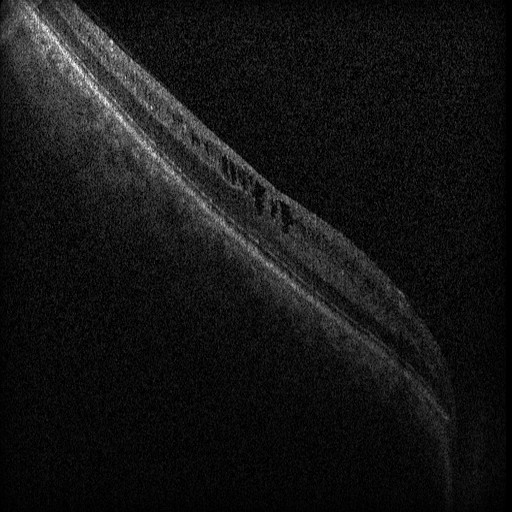 OCT scan showing DME.